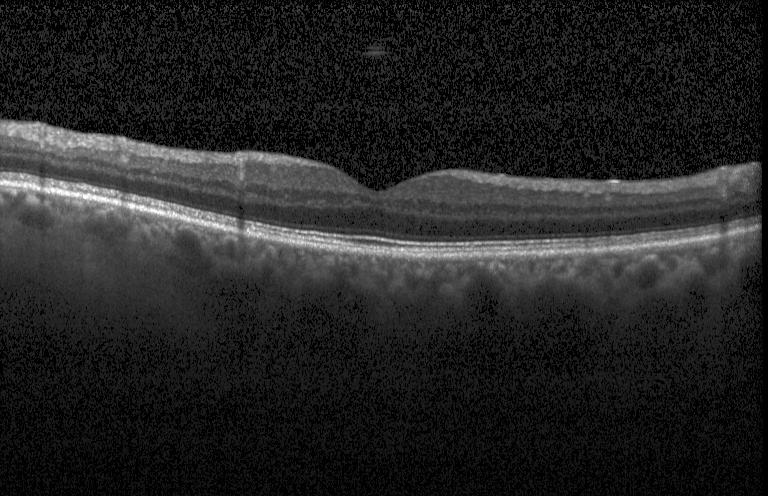

Retinal OCT cross-section; spectral-domain OCT; through the macula; acquired on a Heidelberg Spectralis
Dx: no evidence of choroidal neovascularization, diabetic macular edema, or drusen.